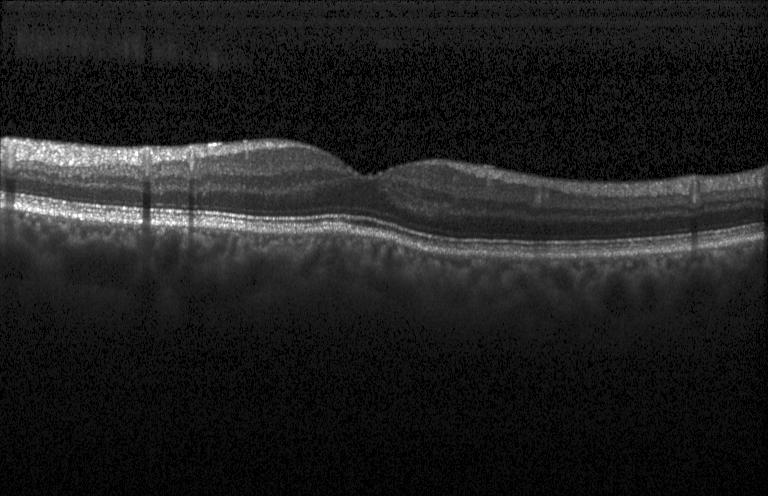
Spectral-domain OCT B-scan: neither CNV, DME, nor drusen.